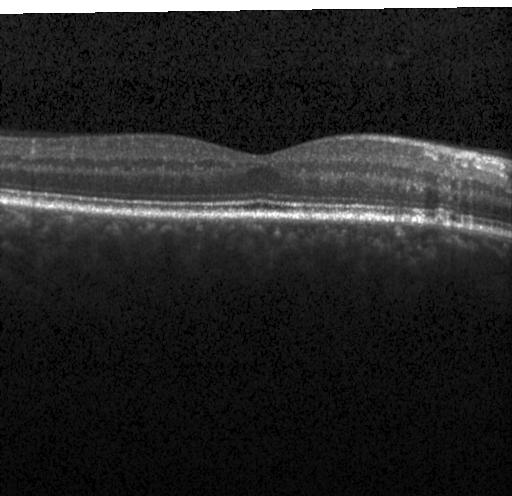 OCT scan showing no evidence of choroidal neovascularization, diabetic macular edema, or drusen.